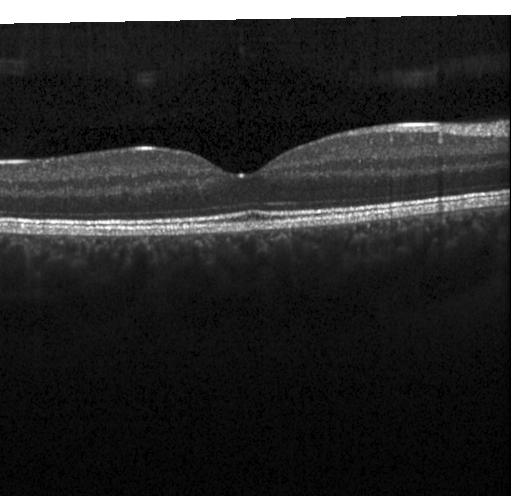

Retinal OCT cross-section.
Diagnosis: no CNV, DME, or drusen.